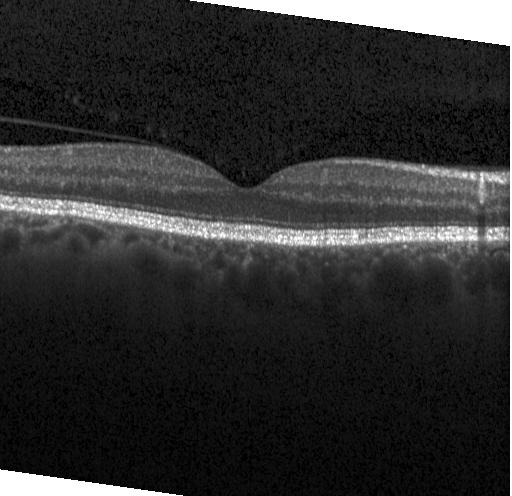
Impression: no CNV, DME, or drusen.